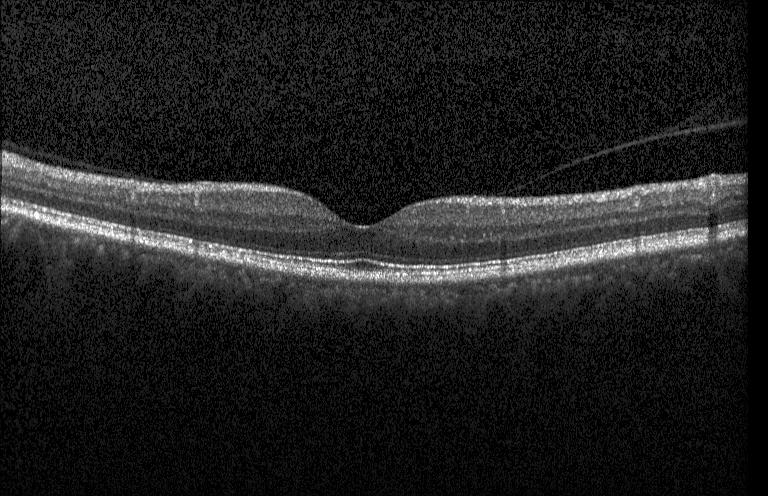 Retinal OCT B-scan. This B-scan demonstrates neither choroidal neovascularization, diabetic macular edema, nor drusen.